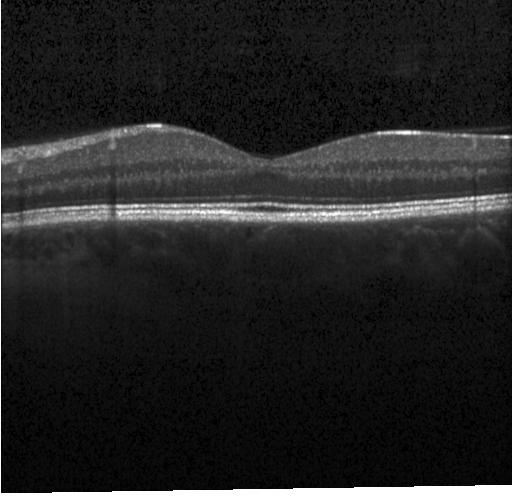
OCT B-scan. OCT finding: neither choroidal neovascularization, diabetic macular edema, nor drusen.